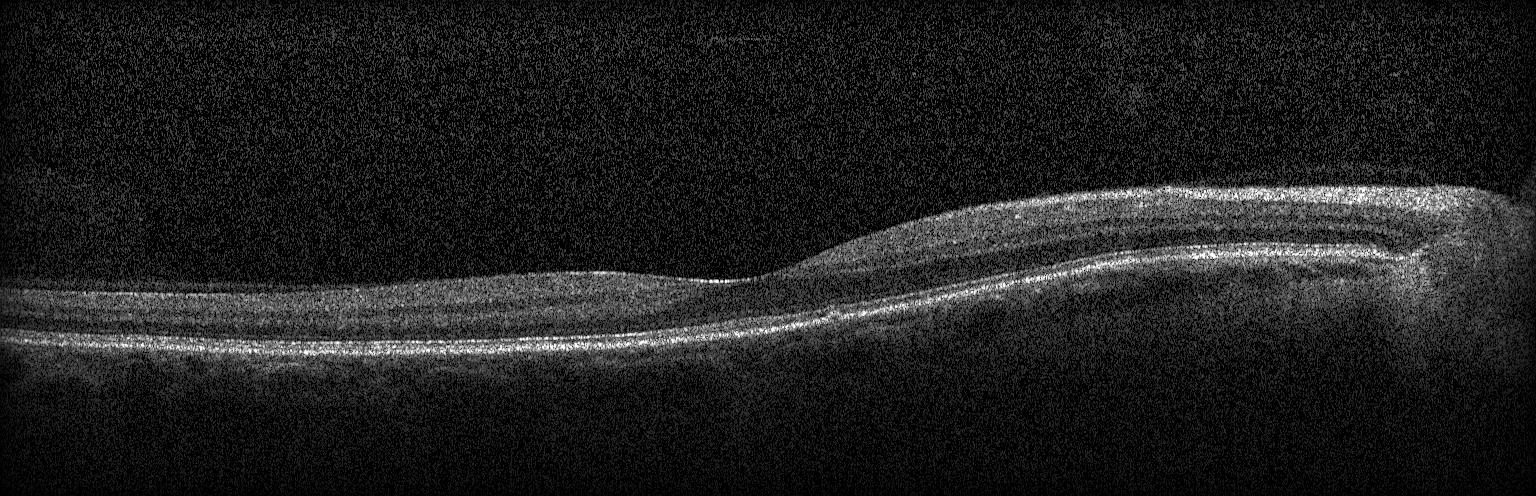

Dx: neither CNV, DME, nor drusen.